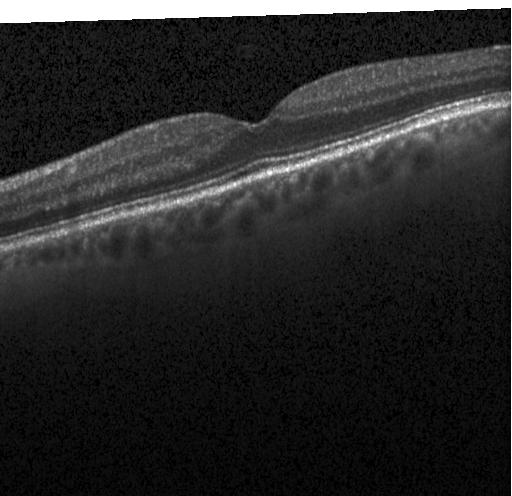 Retinal OCT B-scan — Macular OCT: no choroidal neovascularization, no diabetic macular edema, and no drusen.